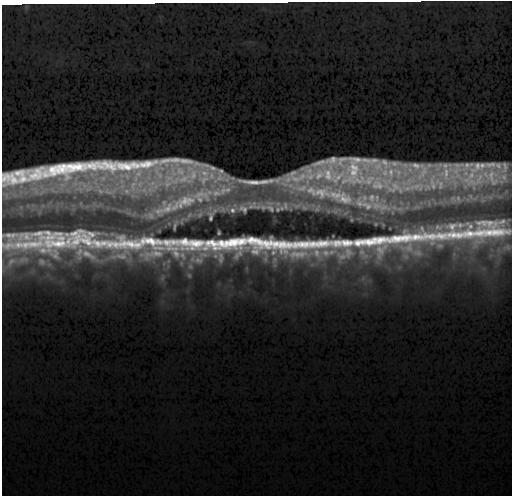 Optical coherence tomography B-scan
Diagnosis: a choroidal neovascular membrane.